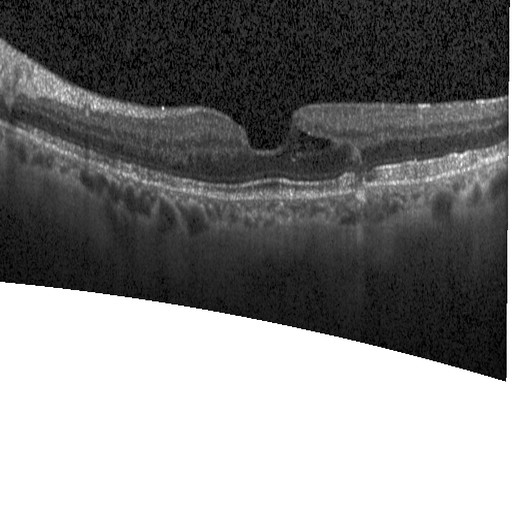

Assessment: diabetic macular edema (DME).